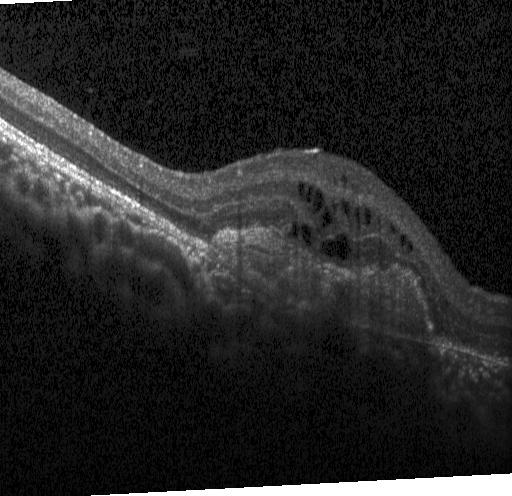
Retinal OCT B-scan. Spectral-domain OCT. Fovea-centered — Diagnosis: CNV.